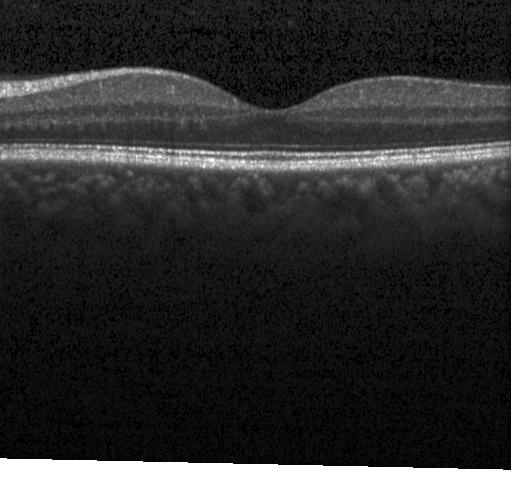 OCT B-scan showing no evidence of choroidal neovascularization, diabetic macular edema, or drusen.